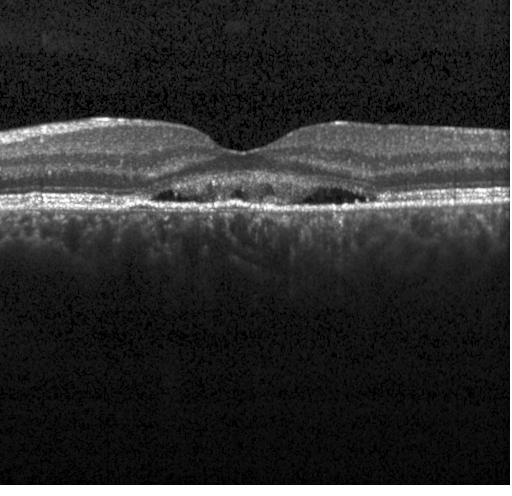

Retinal OCT B-scan.
A choroidal neovascular membrane.